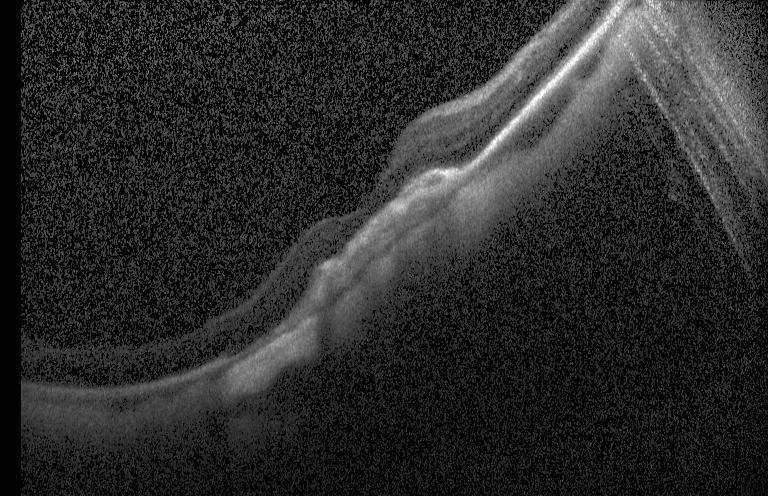 Impression: a choroidal neovascular membrane.